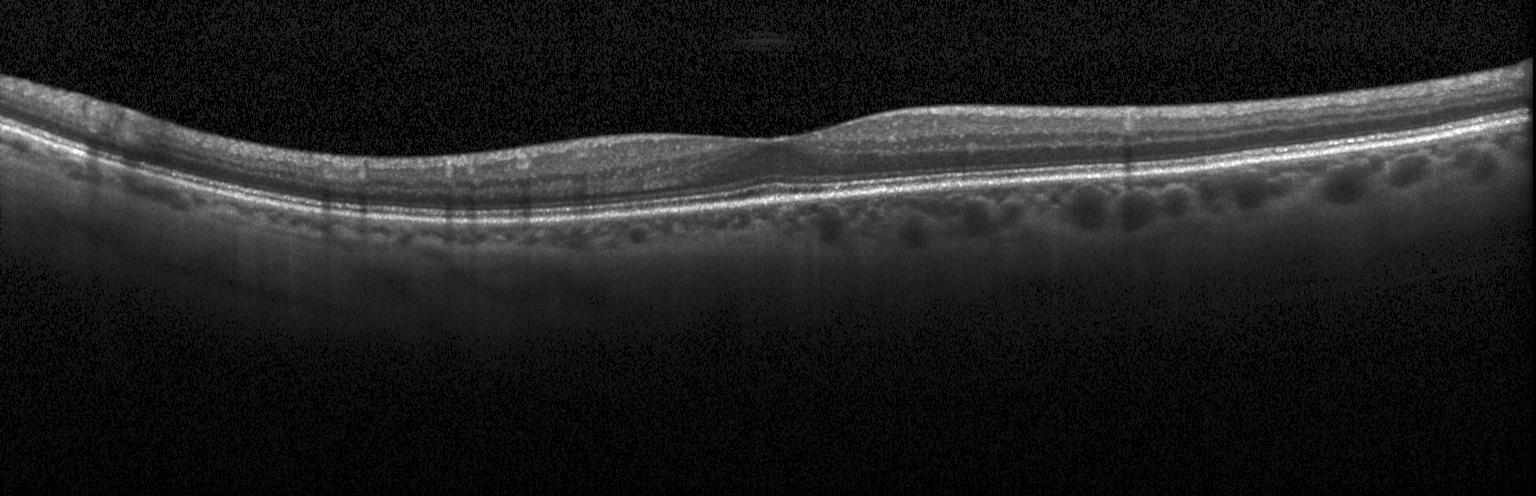

Spectral-domain OCT · OCT line scan · Heidelberg Spectralis OCT system — Neither choroidal neovascularization, diabetic macular edema, nor drusen.